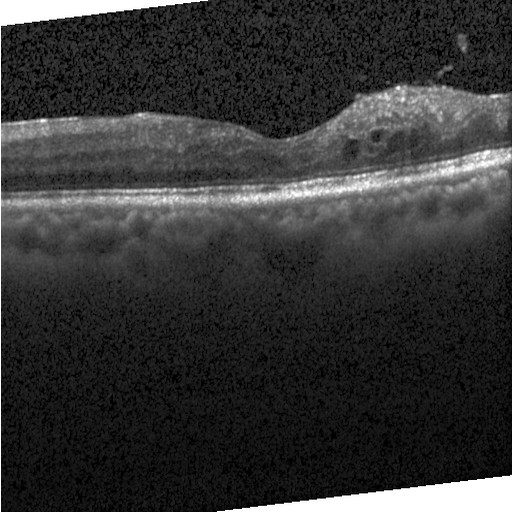

Fovea-centered · Heidelberg Spectralis · SD-OCT · OCT line scan.
The scan shows diabetic macular edema.